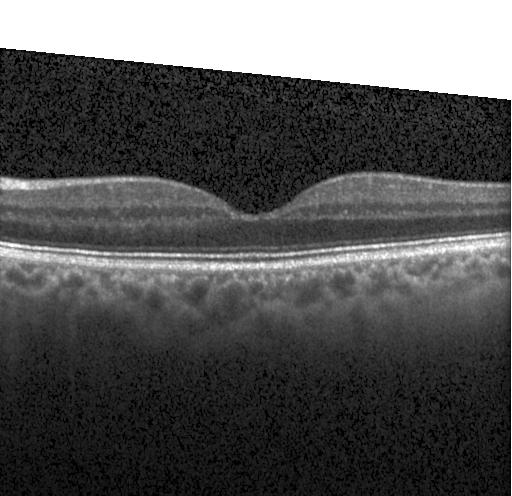

This B-scan demonstrates neither CNV, DME, nor drusen.